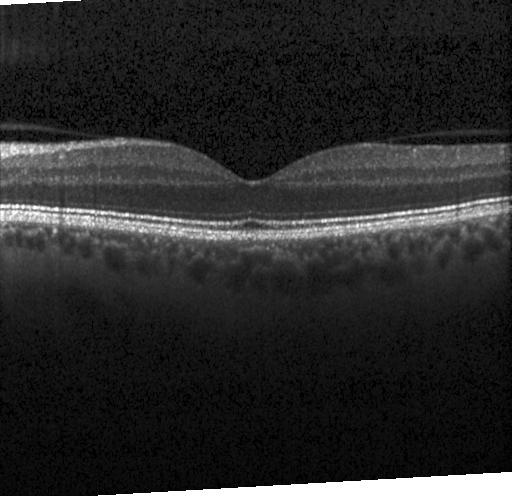

OCT finding: no choroidal neovascularization, no diabetic macular edema, and no drusen.